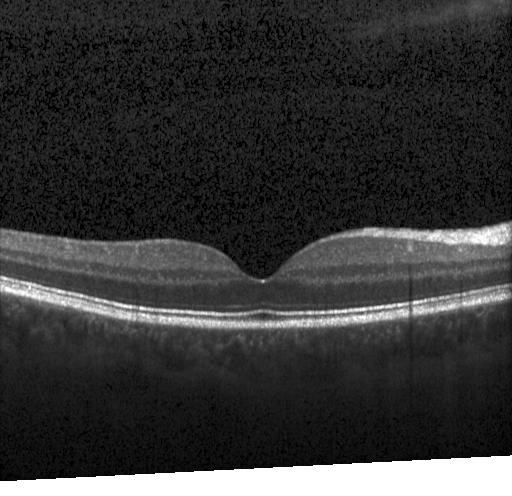 Retinal OCT cross-section showing no evidence of CNV, DME, or drusen.